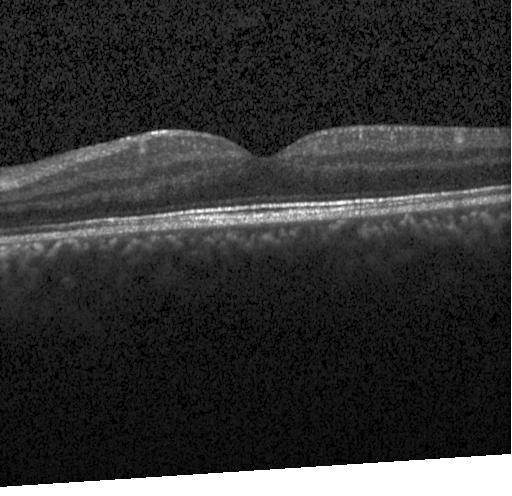
Spectral-domain optical coherence tomography · retinal OCT B-scan · centered on the fovea. Finding: neither choroidal neovascularization, diabetic macular edema, nor drusen.